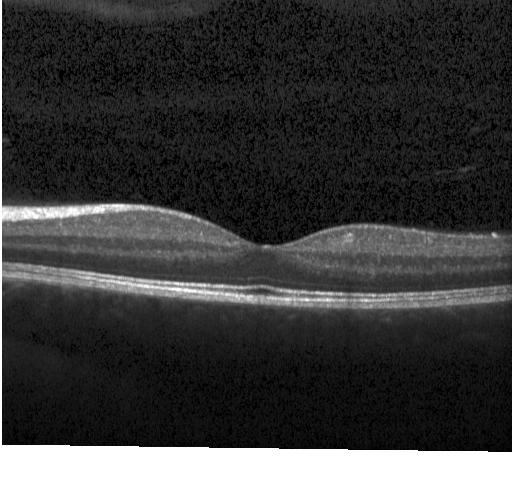

Diagnosis: no choroidal neovascularization, no diabetic macular edema, and no drusen.